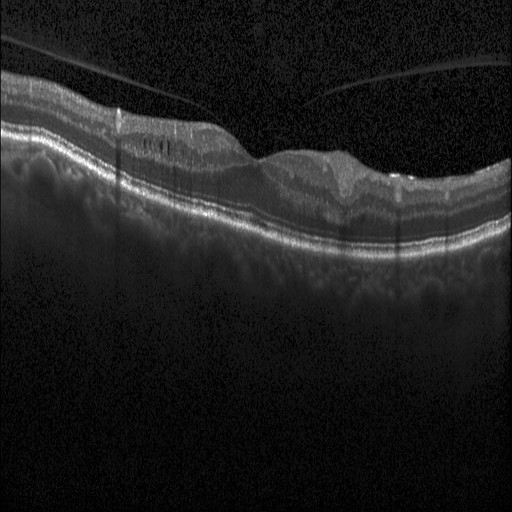
OCT B-scan · horizontal scan through the fovea · Heidelberg Spectralis — Finding: DME.